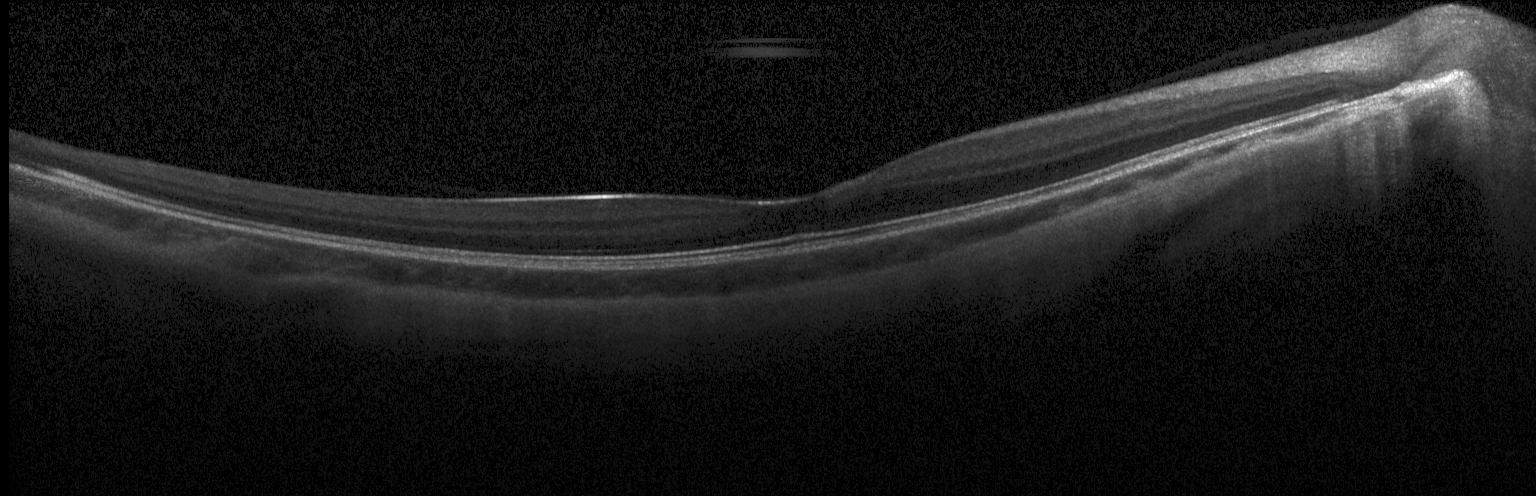
Dx: no choroidal neovascularization, diabetic macular edema, or drusen.